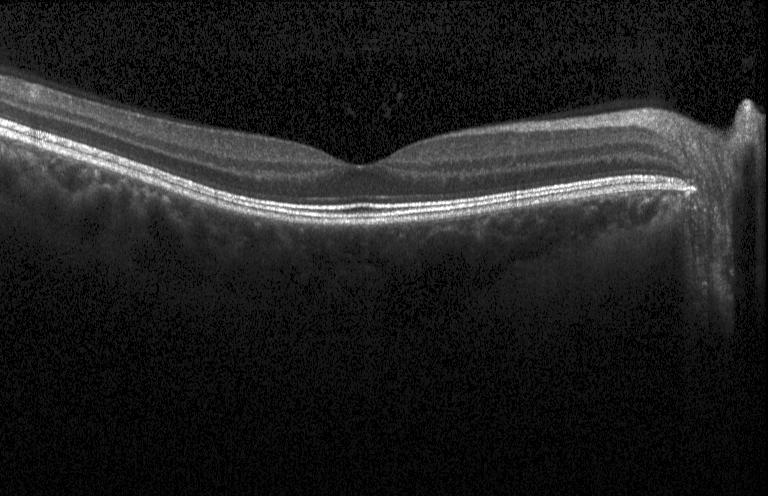
Acquired on a Heidelberg Spectralis · retinal OCT B-scan — Diagnosis: no choroidal neovascularization, no diabetic macular edema, and no drusen.